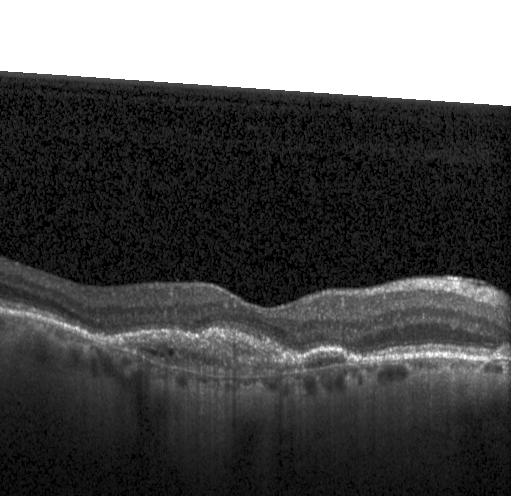 Diagnosis: a choroidal neovascular membrane.